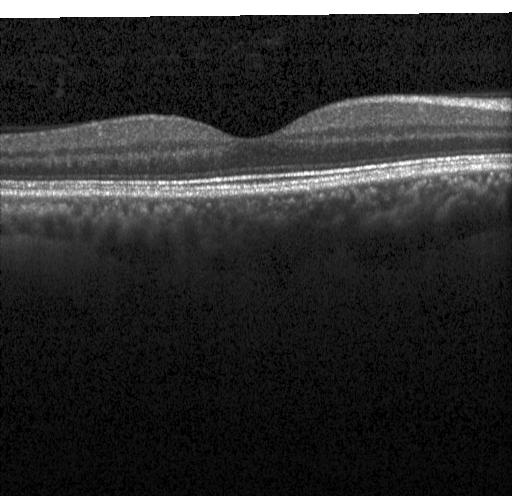 Retinal OCT cross-section — Finding: no evidence of choroidal neovascularization, diabetic macular edema, or drusen.